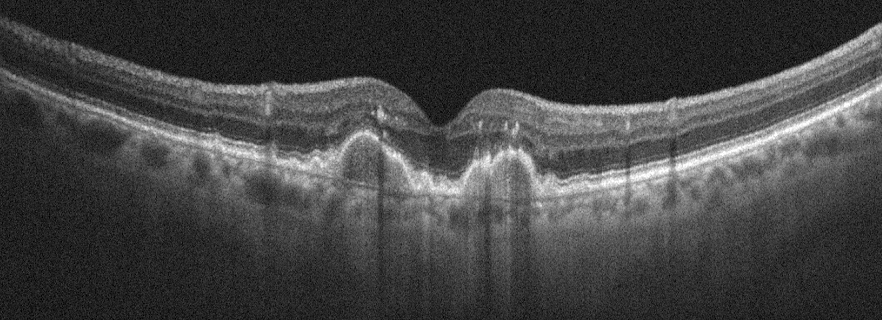

Macular scan. Left eye. OCT line scan. Instrument: Optovue Avanti RTVue XR. Diagnosis: age-related macular degeneration.